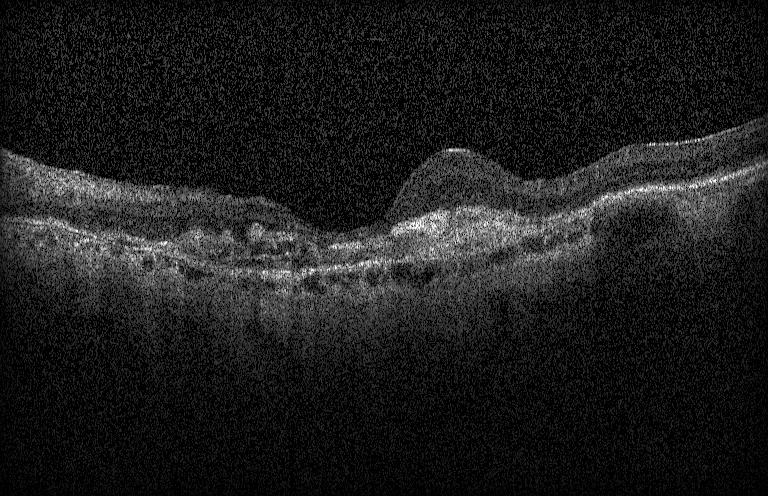 Finding: a choroidal neovascular membrane.